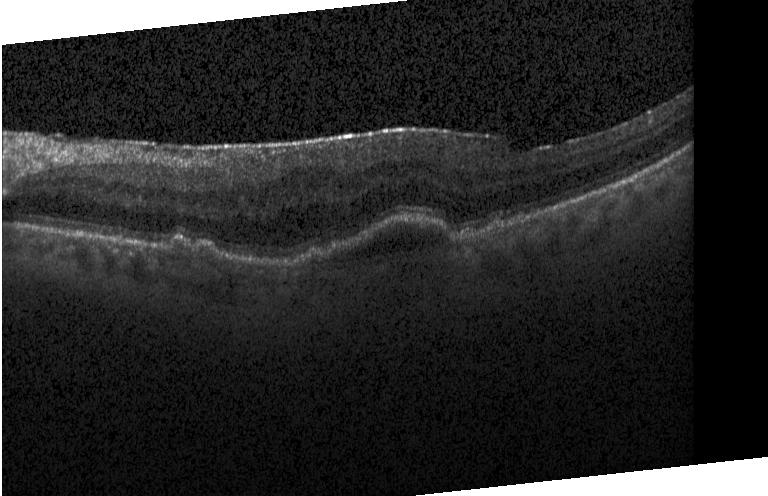

Impression: a choroidal neovascular membrane.